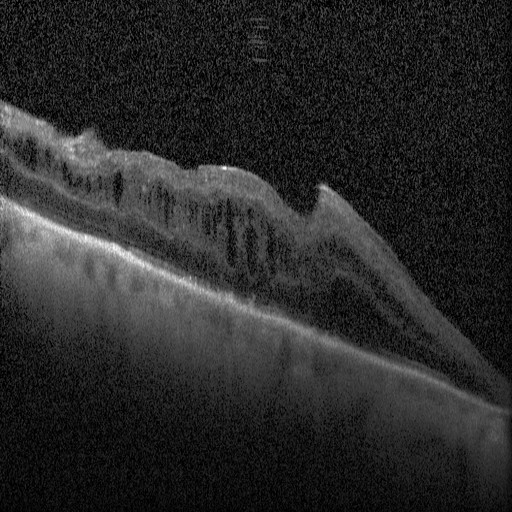

Optical coherence tomography B-scan
Impression: diabetic macular edema.